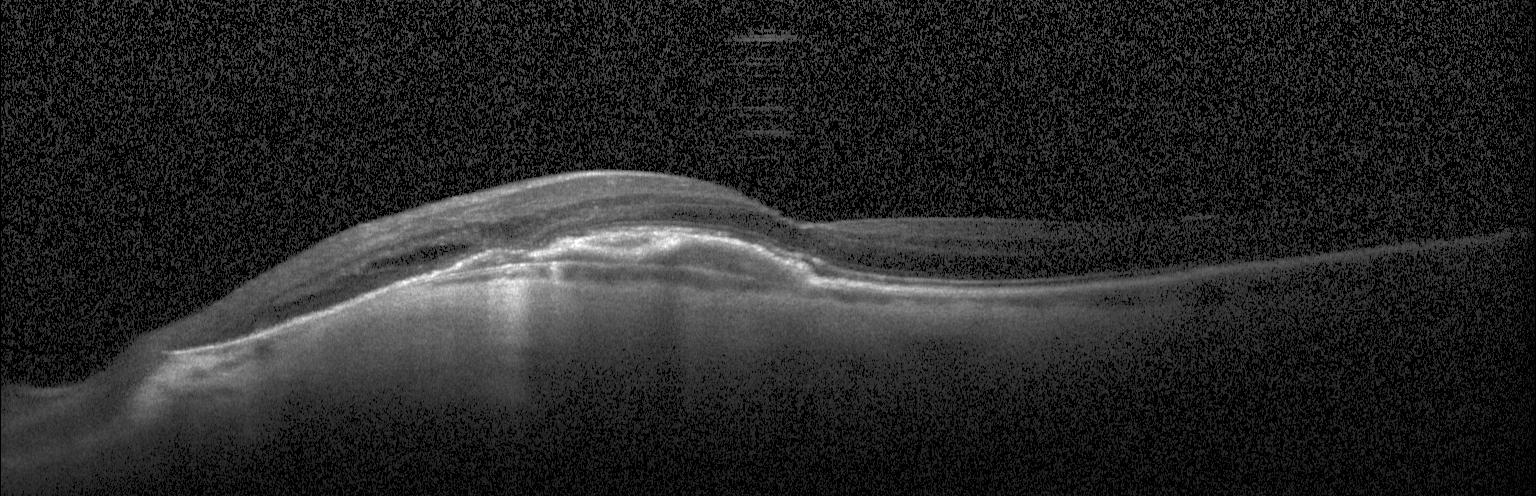

Impression: a choroidal neovascular membrane.